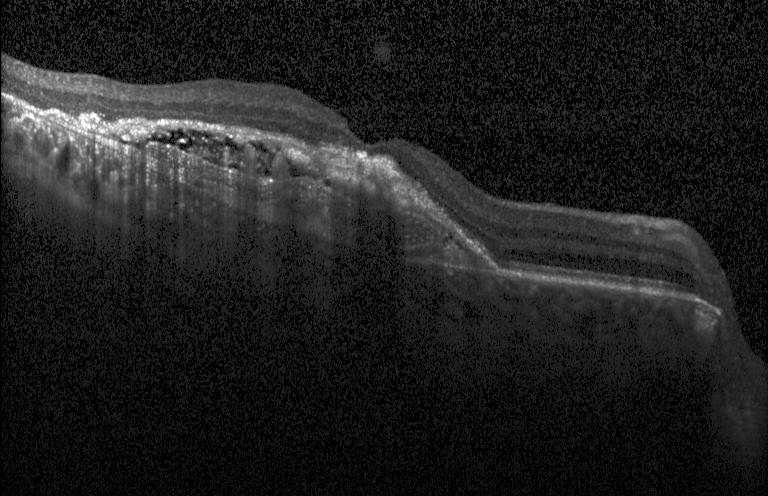
Heidelberg Spectralis · optical coherence tomography scan · spectral-domain OCT
This B-scan demonstrates a choroidal neovascular membrane.